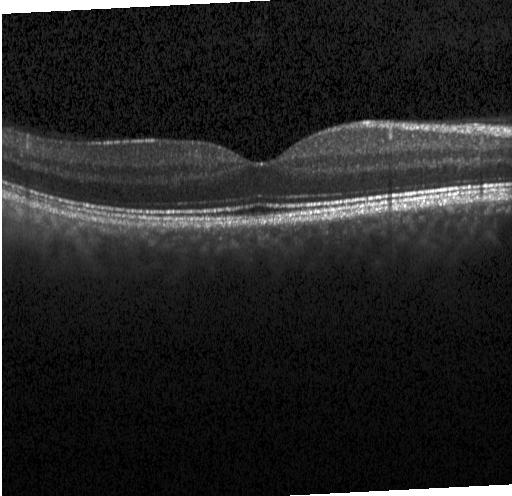 Retinal OCT B-scan — Macular OCT: no choroidal neovascularization, diabetic macular edema, or drusen.